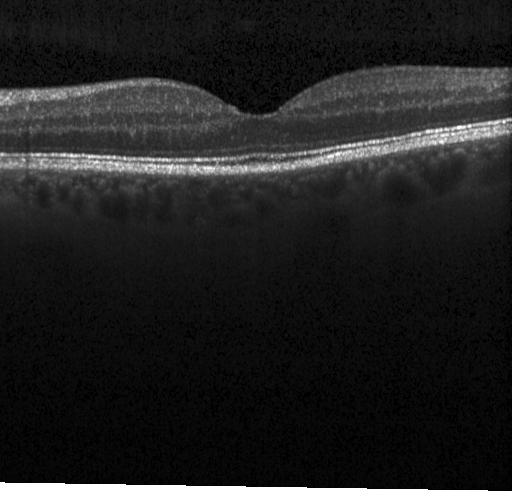

SD-OCT; through the macula; OCT B-scan; instrument: Heidelberg Spectralis. Finding: neither choroidal neovascularization, diabetic macular edema, nor drusen.